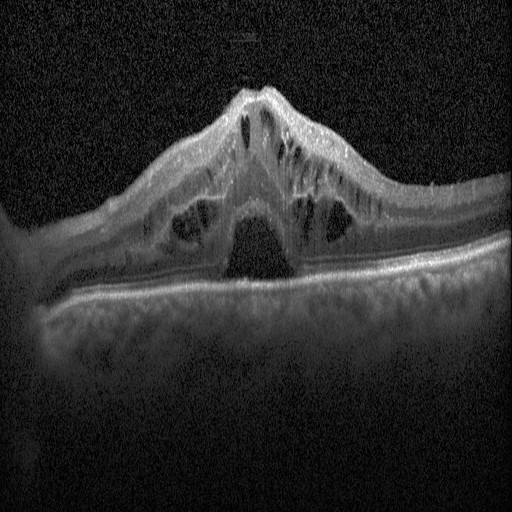 OCT B-scan. Finding: diabetic macular edema.